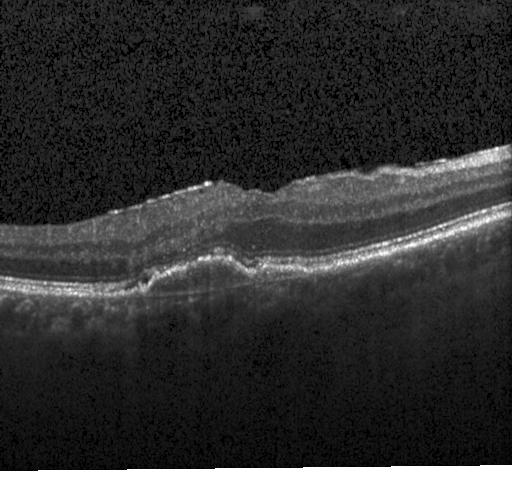

OCT finding: choroidal neovascularization.